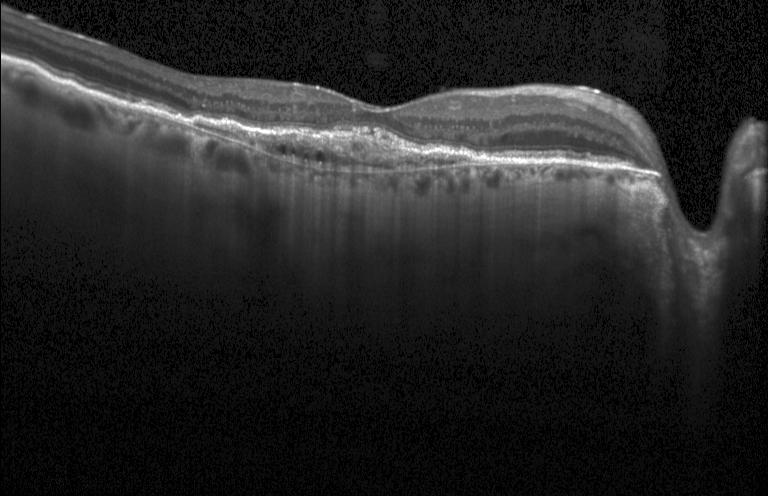 This B-scan demonstrates choroidal neovascularization.